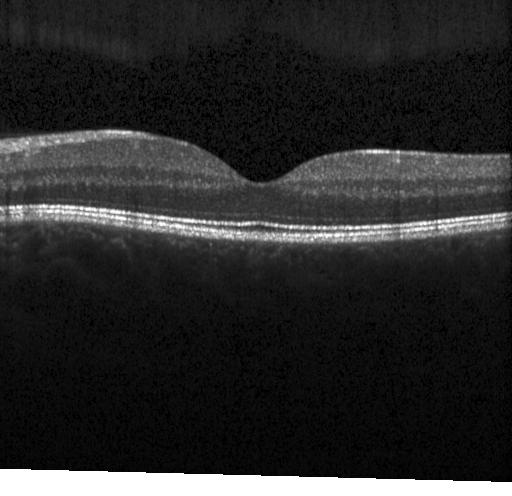

Through the macula. Optical coherence tomography scan. Instrument: Heidelberg Spectralis — Assessment: neither CNV, DME, nor drusen.